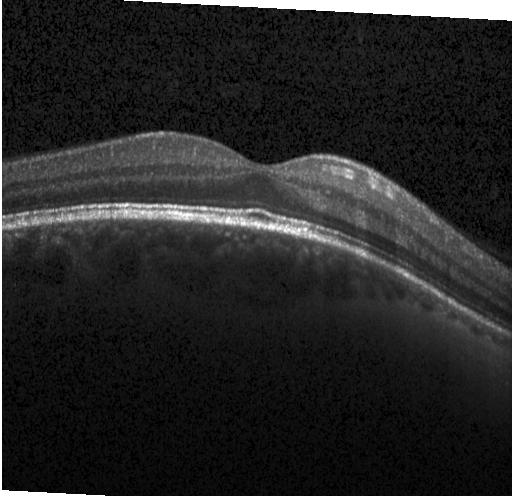

OCT finding: no CNV, DME, or drusen.